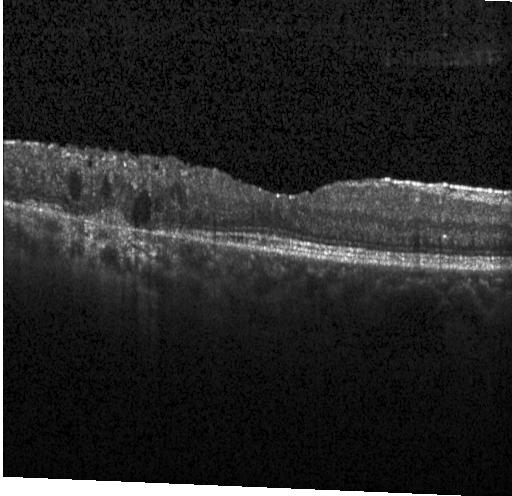 OCT B-scan — Diabetic macular edema.